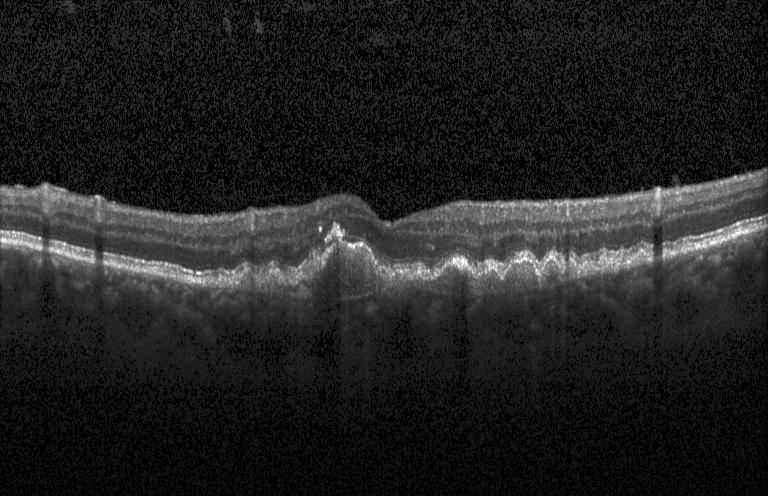
Diagnosis: a choroidal neovascular membrane.